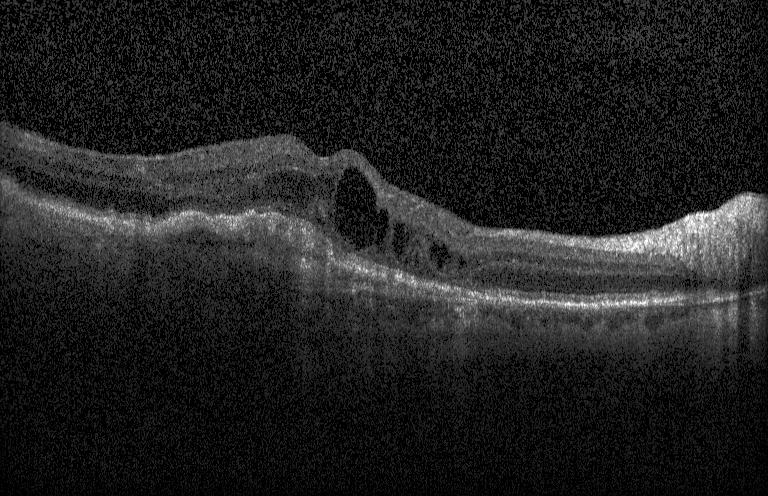 SD-OCT. OCT line scan — A choroidal neovascular membrane.